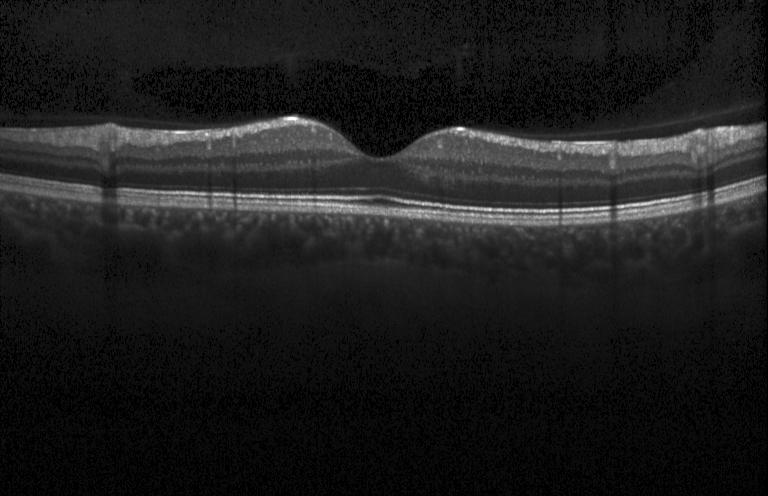
Fovea-centered · spectral-domain optical coherence tomography · retinal OCT cross-section
Diagnosis: neither choroidal neovascularization, diabetic macular edema, nor drusen.